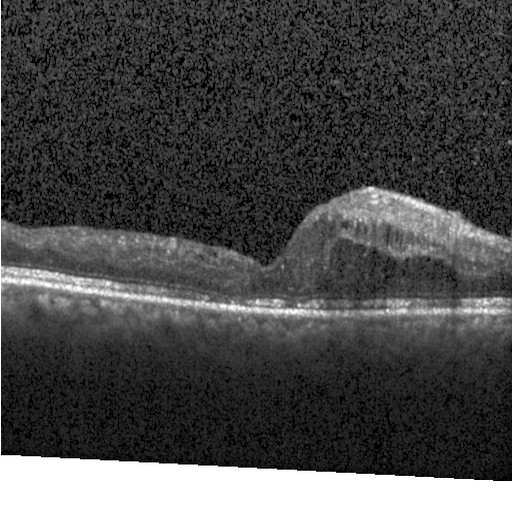
Finding: DME.